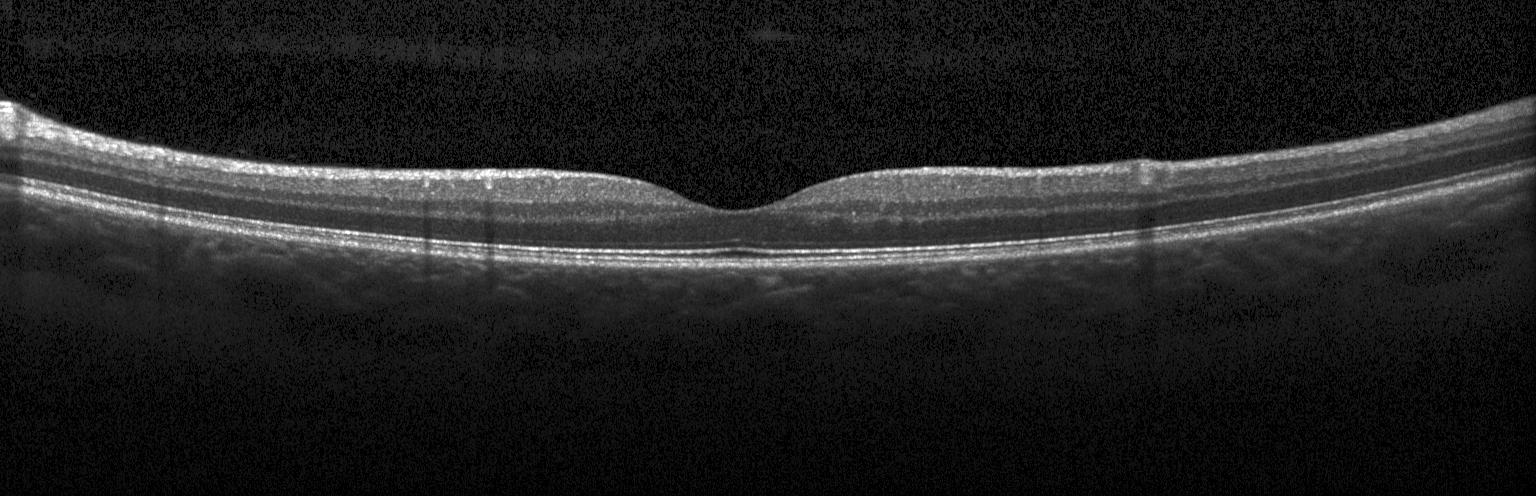 OCT finding: no choroidal neovascularization, diabetic macular edema, or drusen.